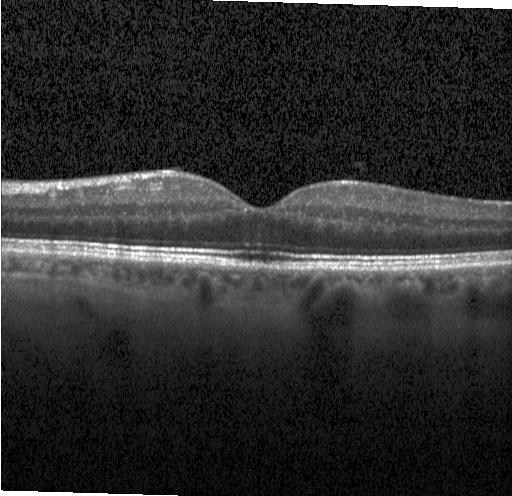

Retinal OCT B-scan; macular scan; acquired on a Heidelberg Spectralis — Finding: neither choroidal neovascularization, diabetic macular edema, nor drusen.